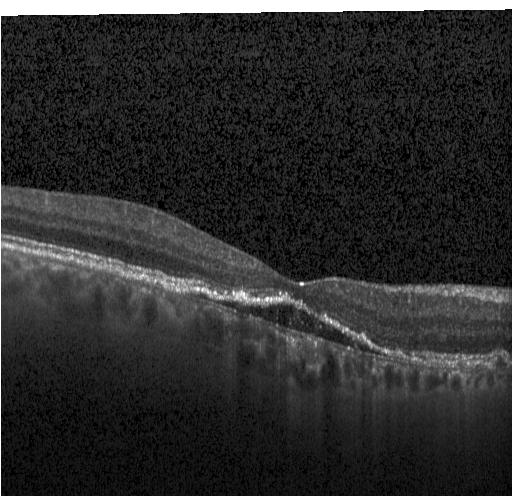 Spectral-domain OCT B-scan: a choroidal neovascular membrane.